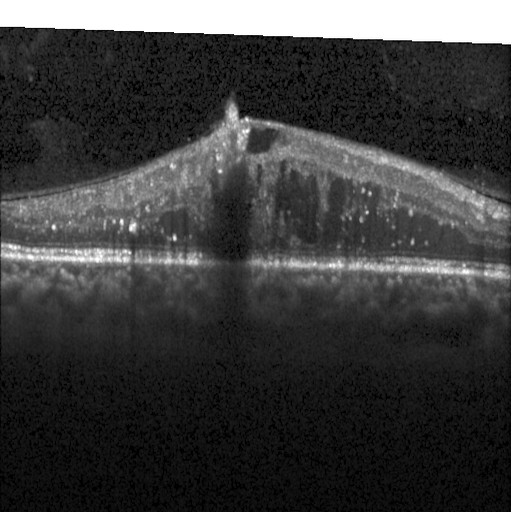
OCT B-scan showing DME.